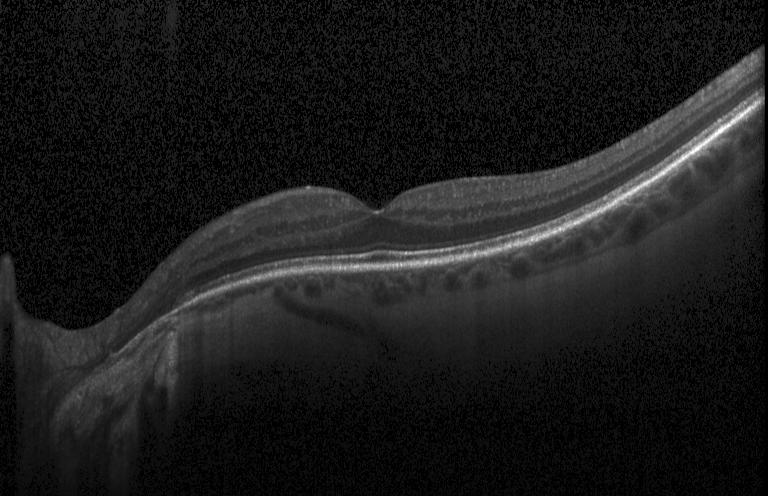
Instrument: Heidelberg Spectralis; OCT line scan
Finding: no choroidal neovascularization, diabetic macular edema, or drusen.